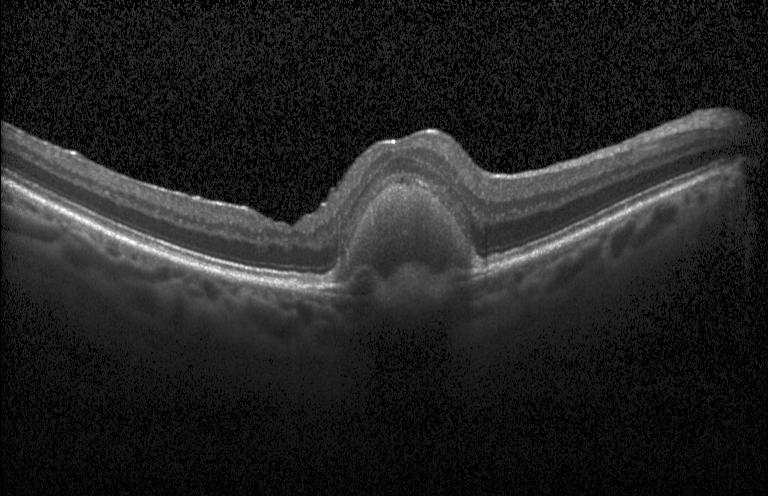
Spectral-domain OCT B-scan: a choroidal neovascular membrane.